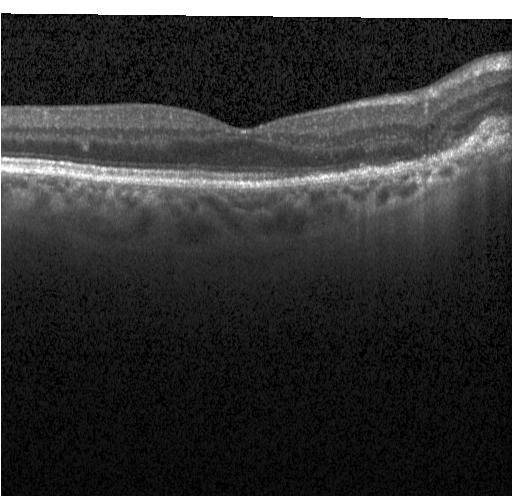 Retinal OCT B-scan; spectral-domain optical coherence tomography — Dx: CNV.